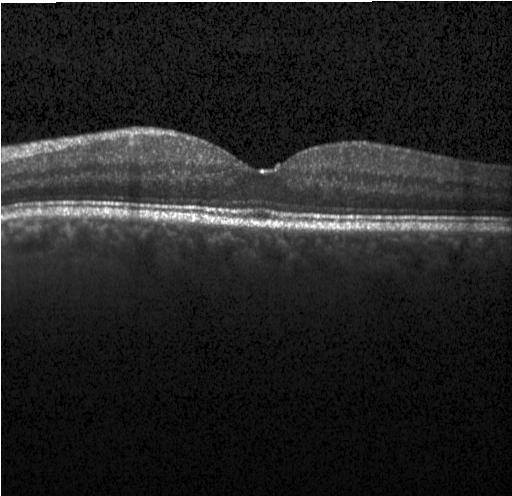

OCT scan showing no choroidal neovascularization, no diabetic macular edema, and no drusen.